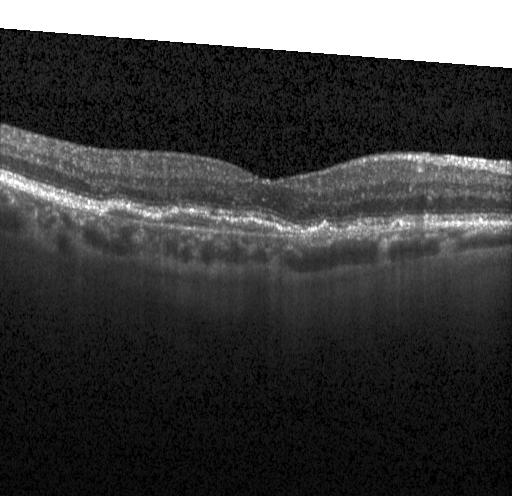 Retinal OCT cross-section
Choroidal neovascularization.